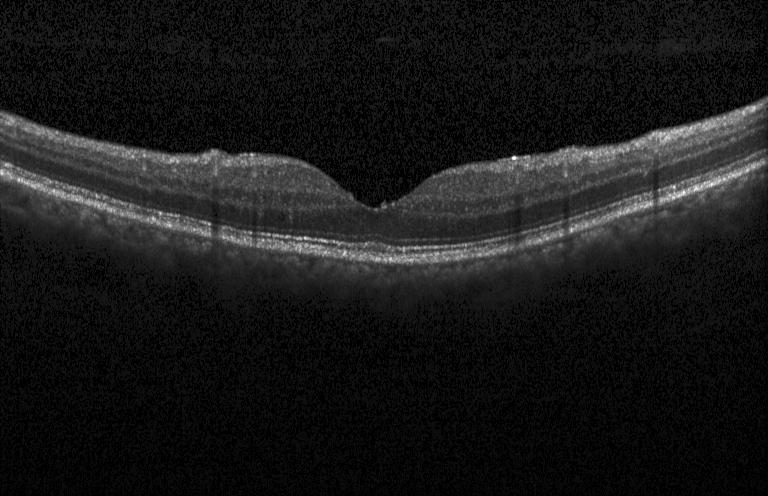

OCT line scan · SD-OCT.
Finding: no evidence of choroidal neovascularization, diabetic macular edema, or drusen.